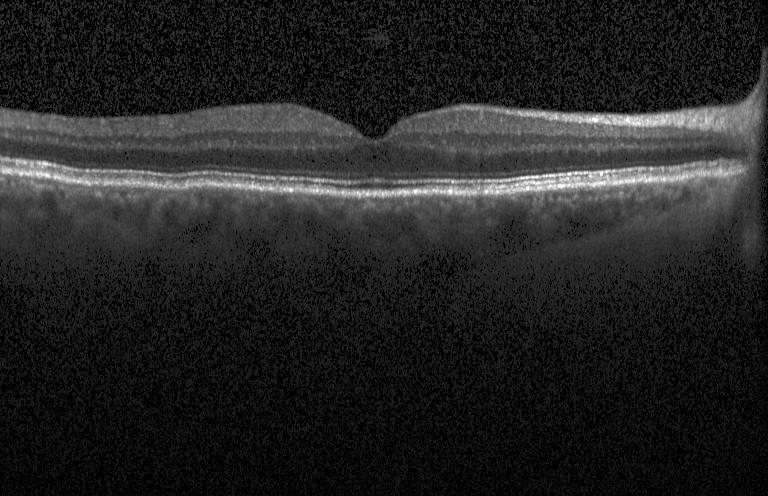

Optical coherence tomography B-scan, instrument: Heidelberg Spectralis, spectral-domain optical coherence tomography. OCT finding: neither CNV, DME, nor drusen.